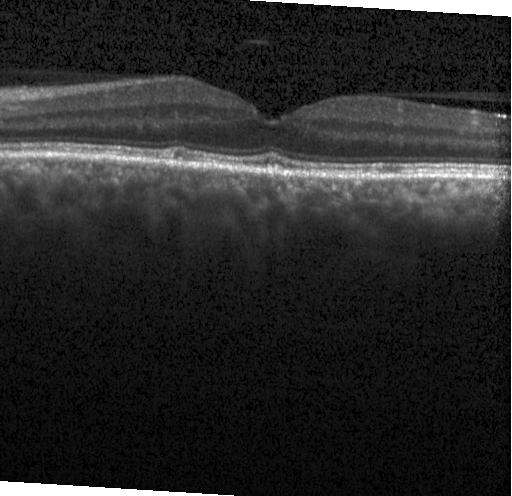 Centered on the fovea. Retinal OCT B-scan.
Assessment: multiple drusen.